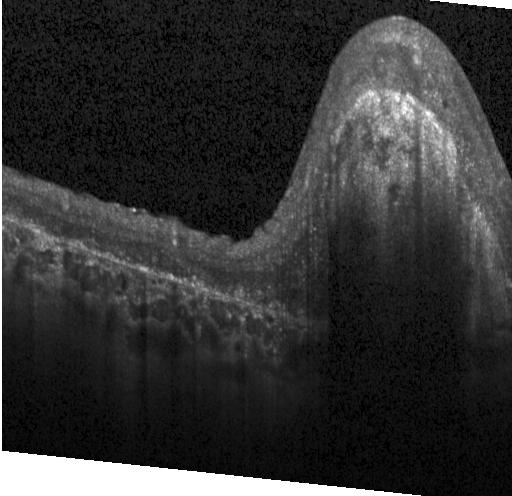 SD-OCT; retinal OCT cross-section; acquired on a Heidelberg Spectralis.
Diagnosis: choroidal neovascularization (CNV).